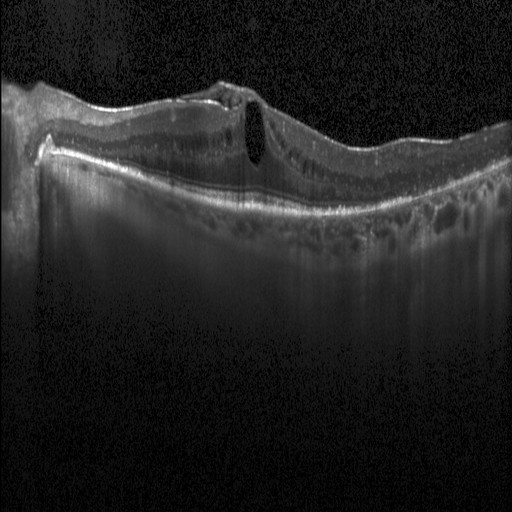

Macular OCT: DME.